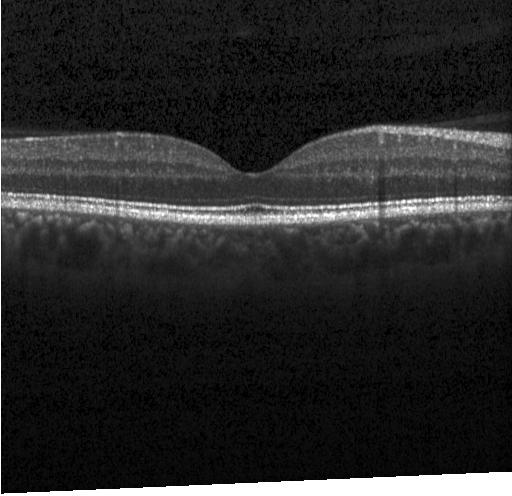 OCT line scan, centered on the fovea — The scan shows neither choroidal neovascularization, diabetic macular edema, nor drusen.